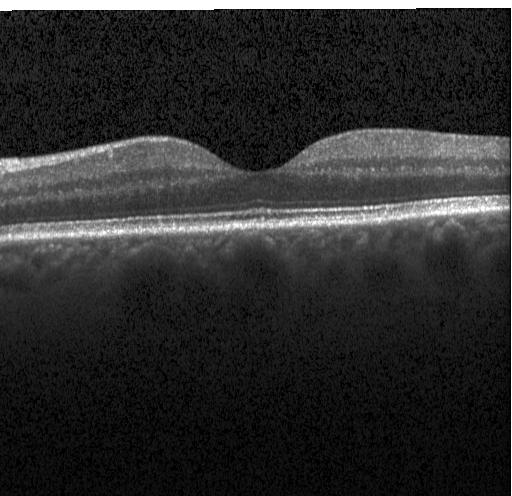
OCT B-scan showing no CNV, no DME, and no drusen.